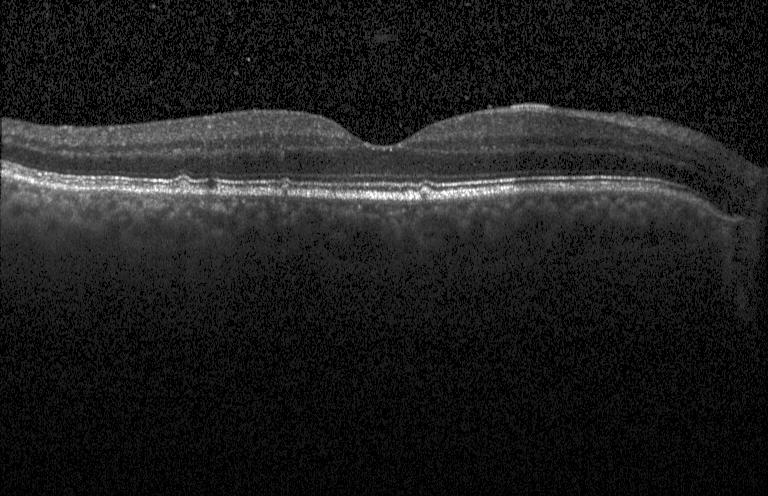
Instrument: Heidelberg Spectralis · OCT B-scan · spectral-domain OCT · centered on the fovea
The scan shows sub-RPE drusenoid deposits.